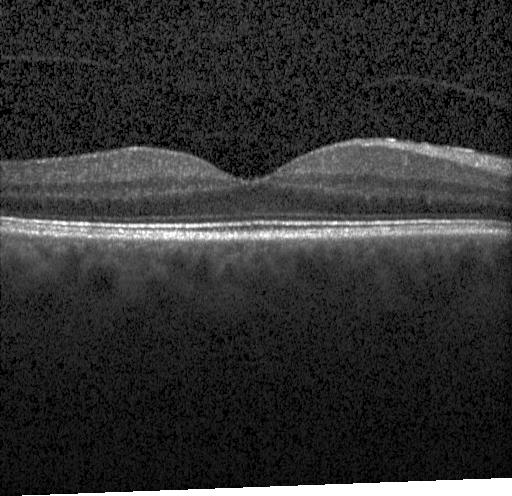

Finding: no CNV, DME, or drusen.